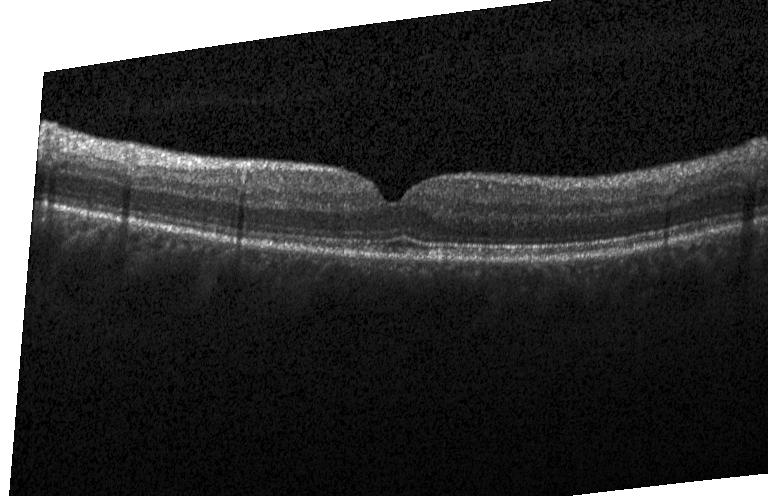 OCT scan showing no choroidal neovascularization, no diabetic macular edema, and no drusen.